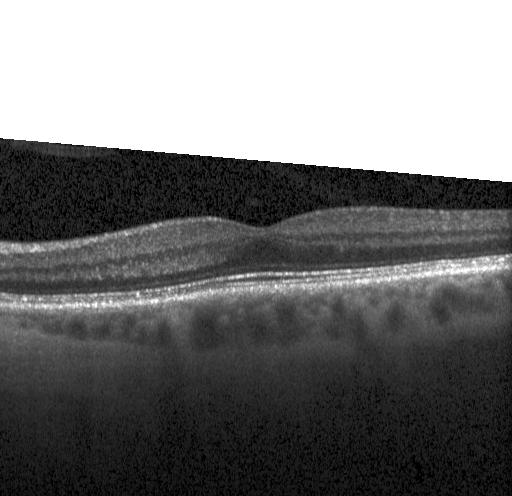

Heidelberg Spectralis OCT system, retinal OCT B-scan. OCT finding: no choroidal neovascularization, diabetic macular edema, or drusen.